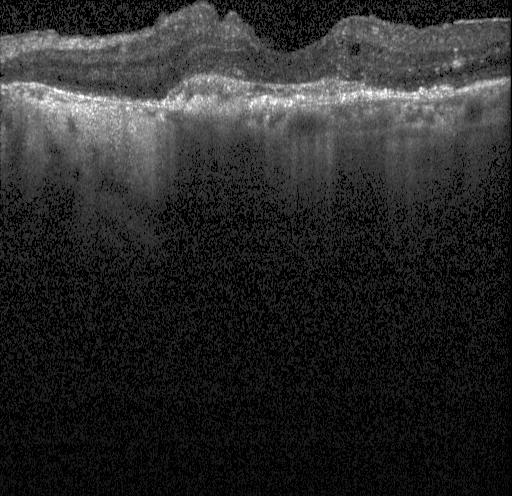

Optical coherence tomography scan. Macular OCT: a choroidal neovascular membrane.